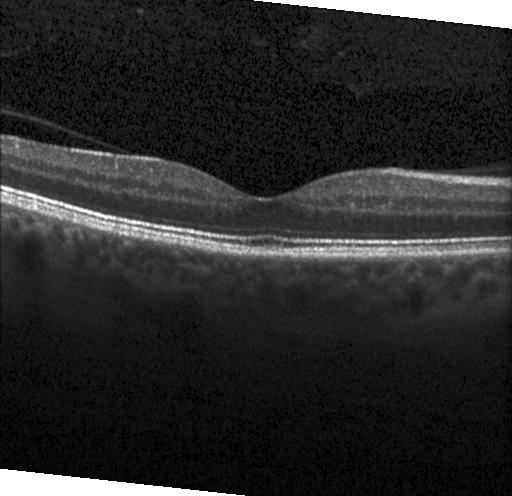 Optical coherence tomography B-scan; centered on the fovea
Neither CNV, DME, nor drusen.